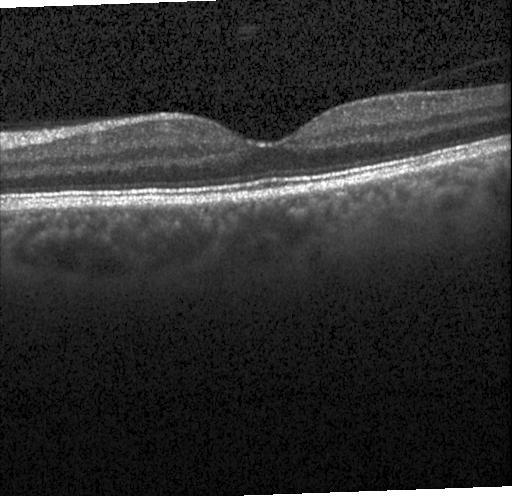
Impression: neither choroidal neovascularization, diabetic macular edema, nor drusen.